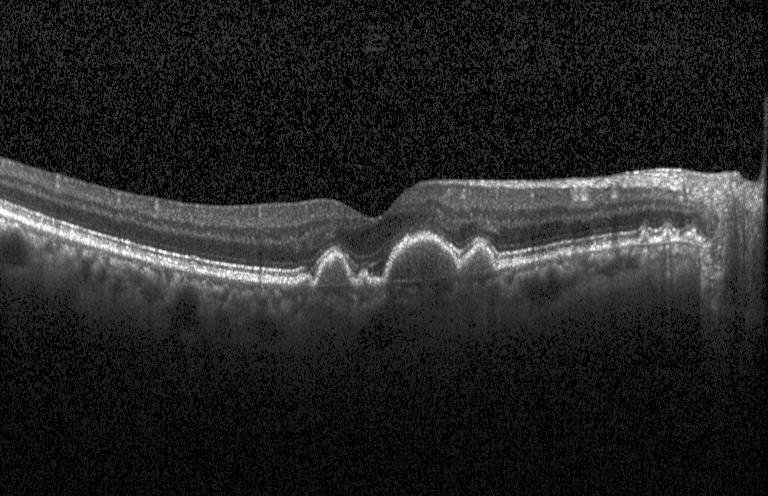 OCT B-scan
Impression: sub-RPE drusenoid deposits.